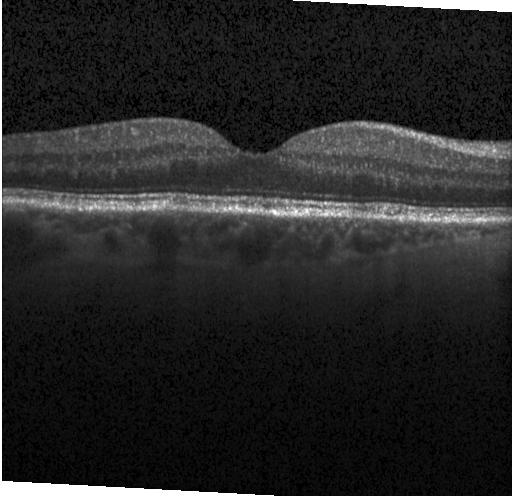
OCT scan showing neither CNV, DME, nor drusen.